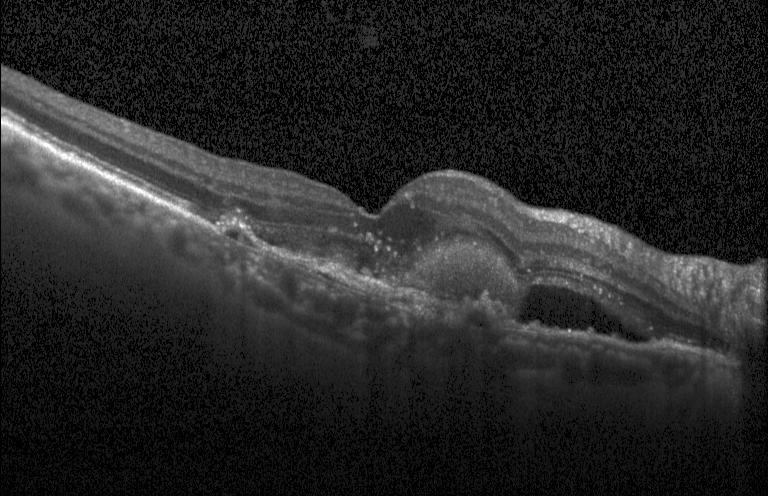
Impression: choroidal neovascularization.